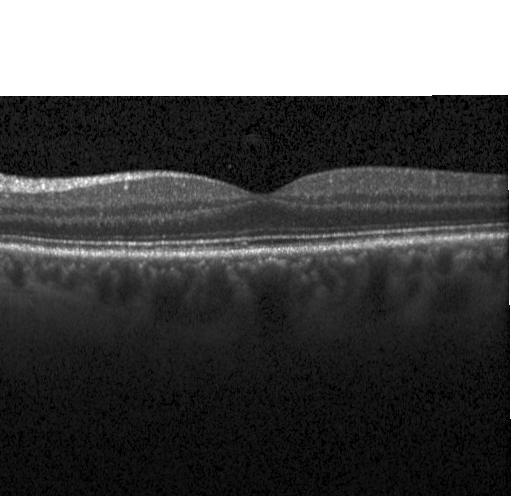

Centered on the fovea; acquired on a Heidelberg Spectralis; spectral-domain OCT; OCT B-scan.
Finding: neither CNV, DME, nor drusen.